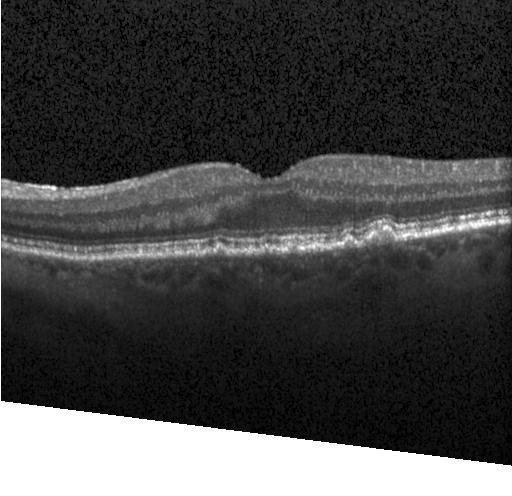

Retinal OCT B-scan. Multiple drusen.